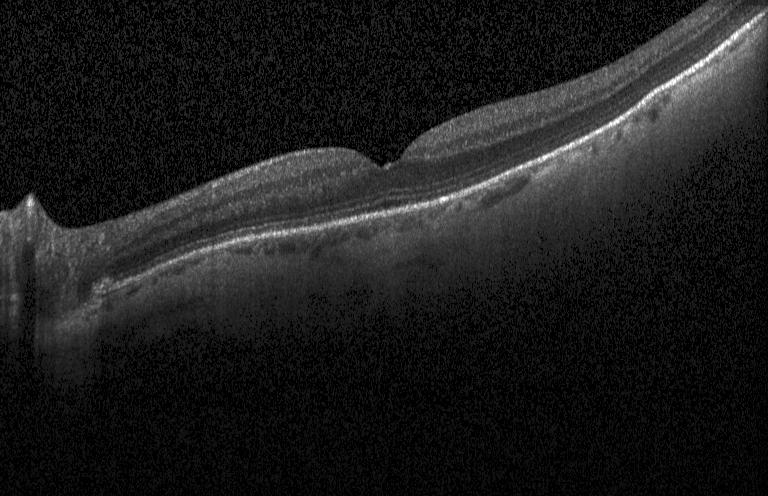
Retinal OCT cross-section.
Neither CNV, DME, nor drusen.